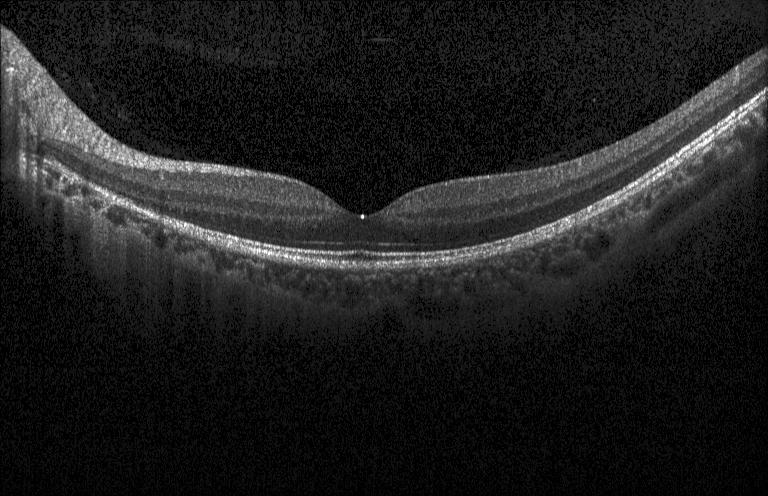
Diagnosis: no choroidal neovascularization, no diabetic macular edema, and no drusen.